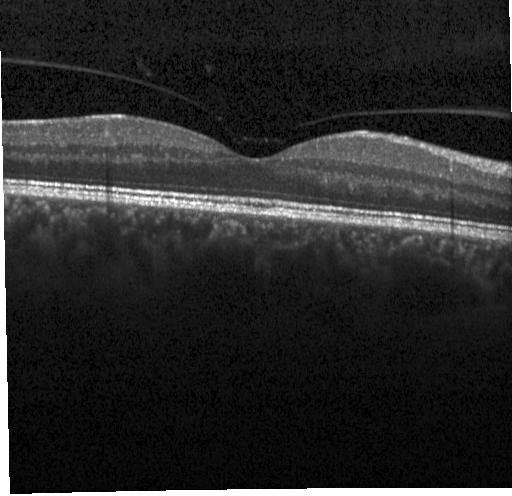

SD-OCT, optical coherence tomography scan — This B-scan demonstrates neither choroidal neovascularization, diabetic macular edema, nor drusen.